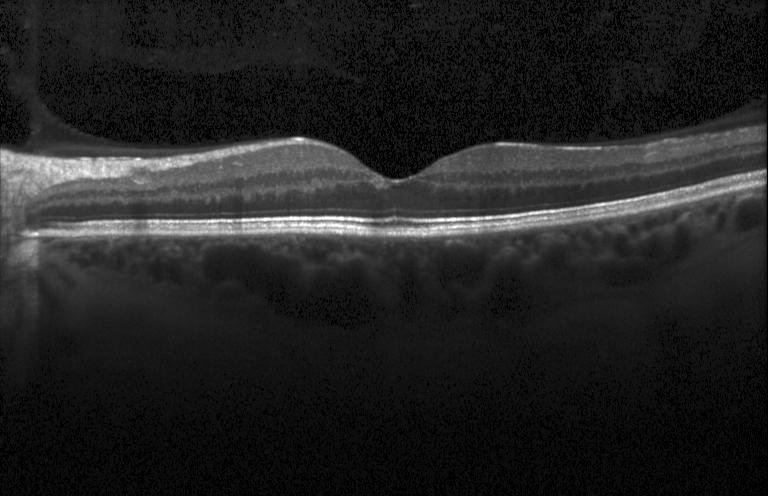
Neither choroidal neovascularization, diabetic macular edema, nor drusen.